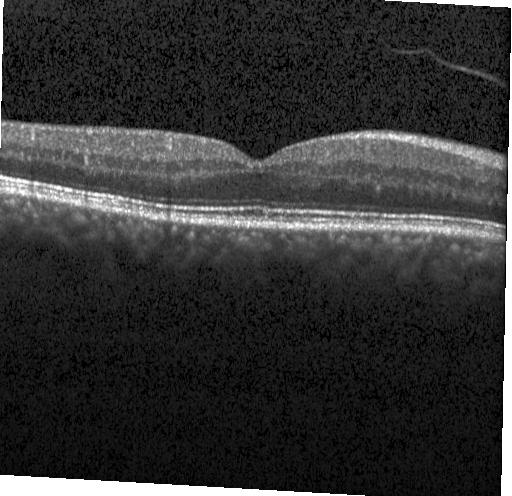 This B-scan demonstrates no evidence of choroidal neovascularization, diabetic macular edema, or drusen.